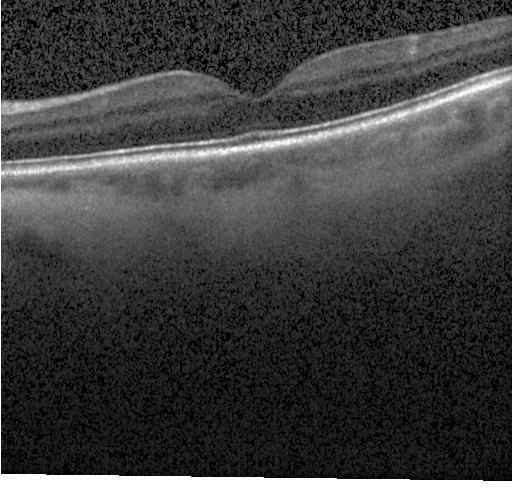 Retinal OCT B-scan; spectral-domain optical coherence tomography.
Dx: no choroidal neovascularization, diabetic macular edema, or drusen.